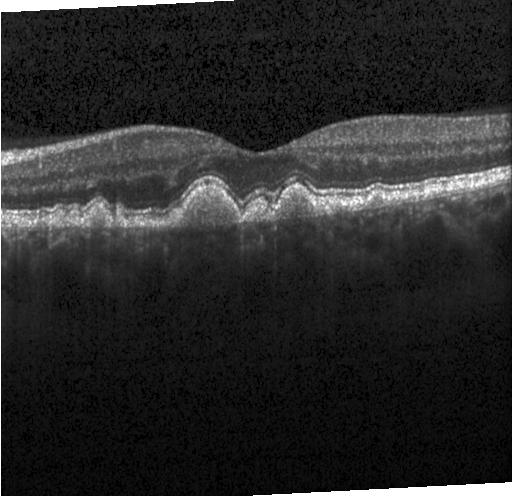
OCT scan showing sub-RPE drusenoid deposits.